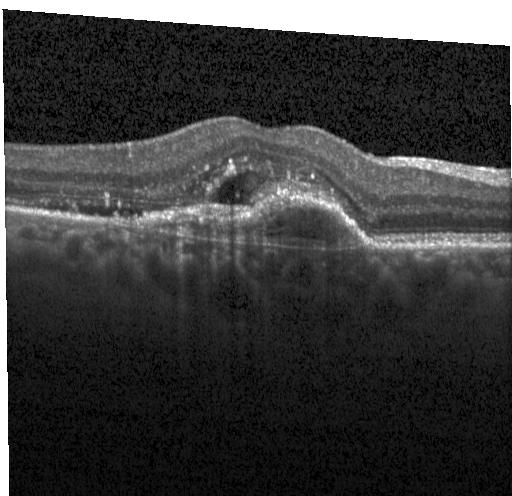
Through the macula; OCT line scan
Diagnosis: a choroidal neovascular membrane.